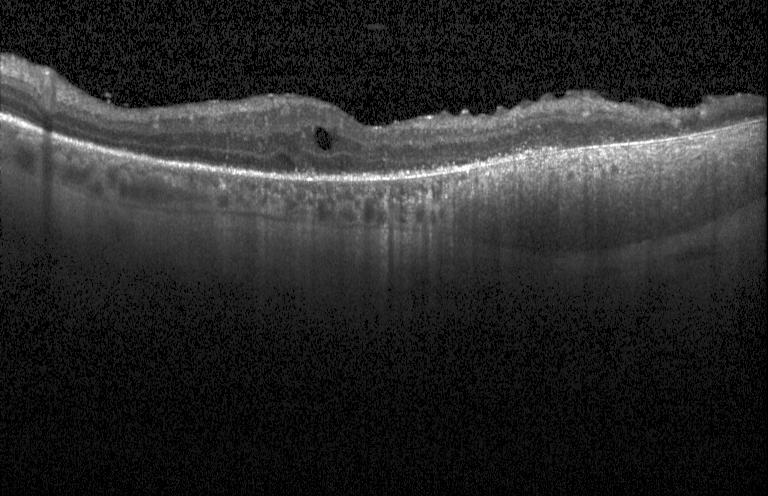

OCT B-scan, SD-OCT.
Diabetic macular edema.